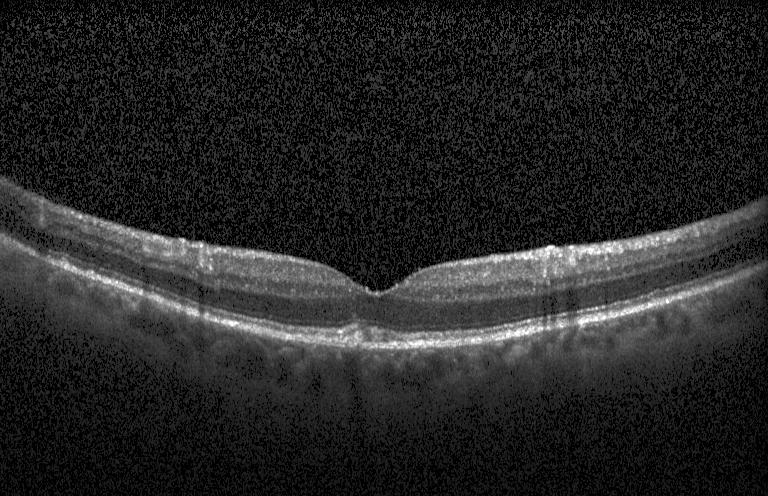
OCT B-scan showing multiple drusen.